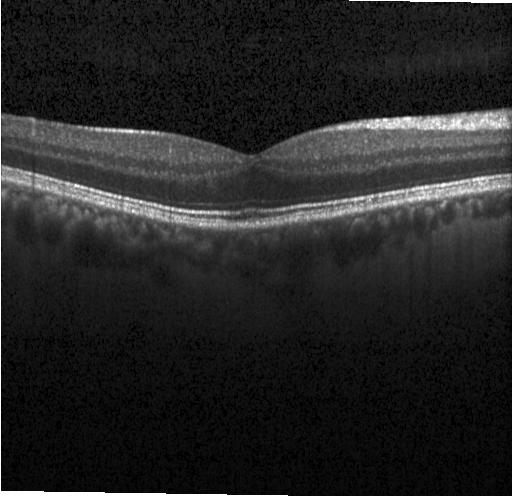
Spectral-domain OCT B-scan: no evidence of CNV, DME, or drusen.